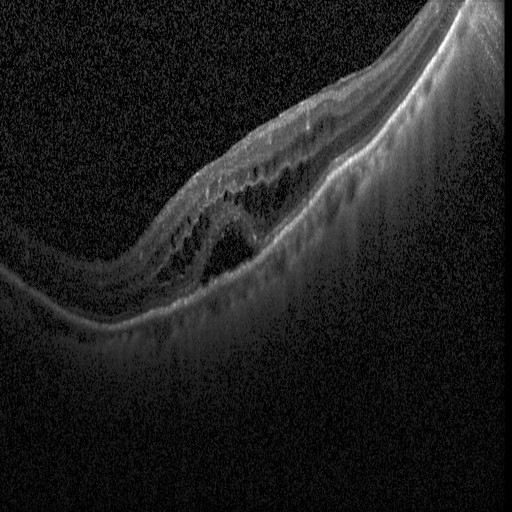 This B-scan demonstrates DME.